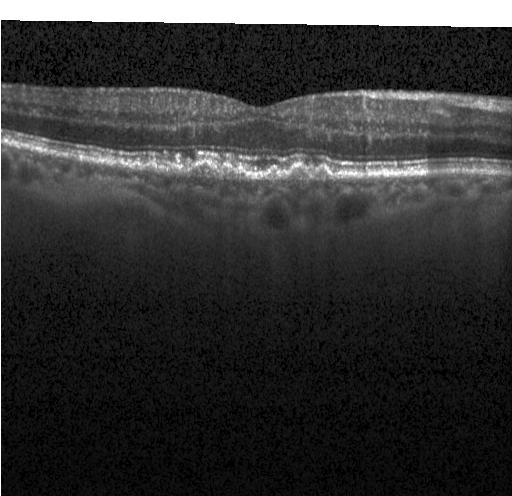

Retinal OCT cross-section.
Impression: multiple drusen.